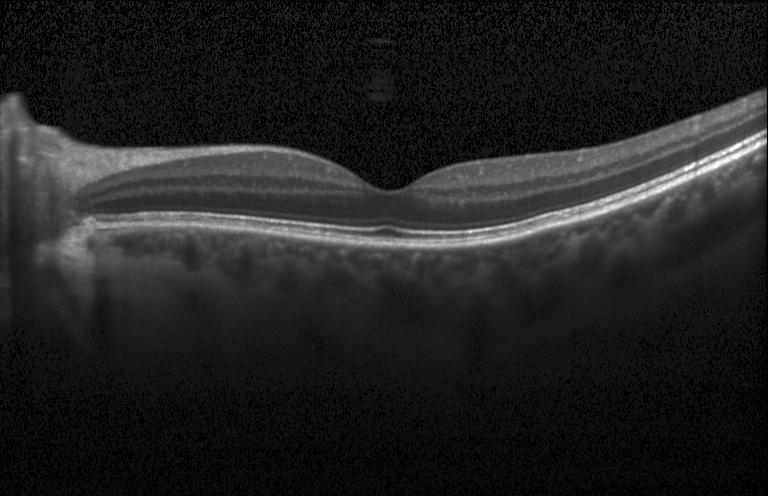

Retinal OCT cross-section showing neither CNV, DME, nor drusen.